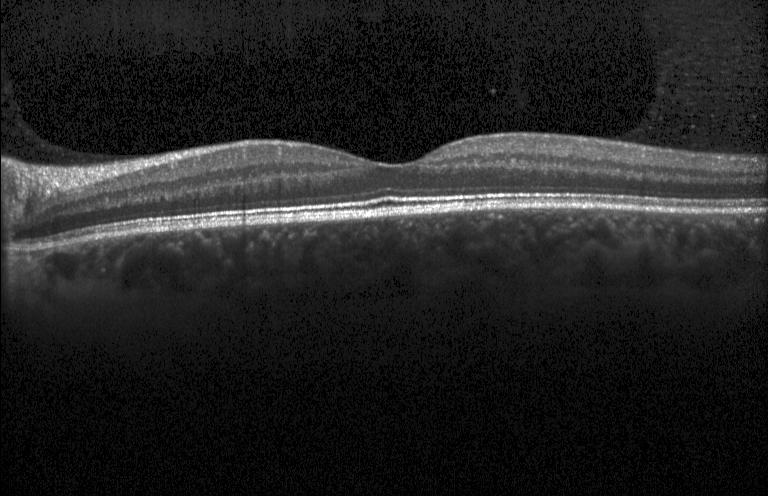 OCT line scan. Finding: no evidence of CNV, DME, or drusen.